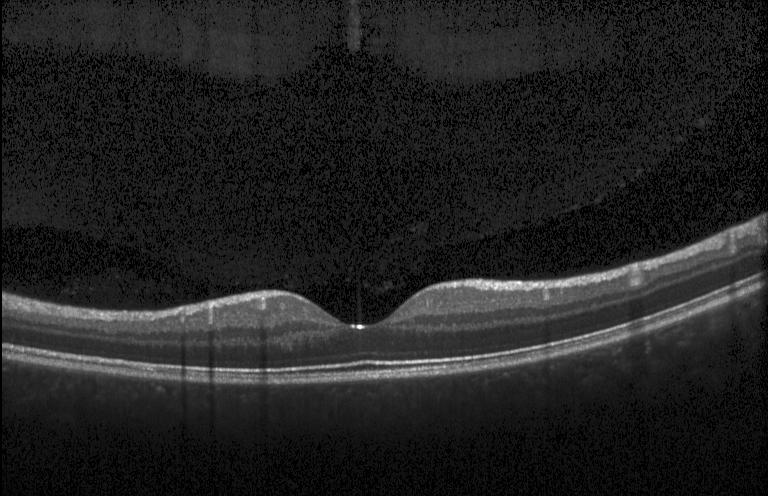 Impression: neither CNV, DME, nor drusen.